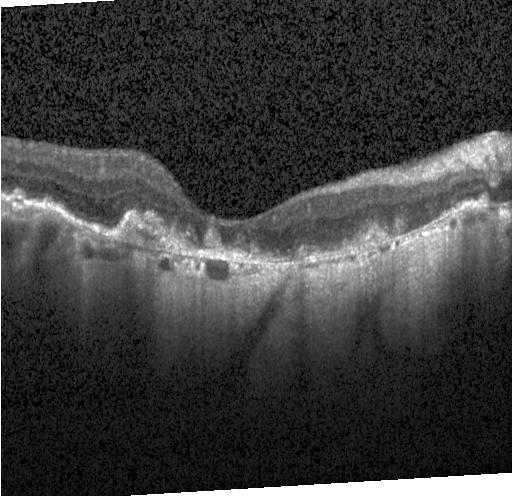 OCT B-scan · instrument: Heidelberg Spectralis · spectral-domain optical coherence tomography. This B-scan demonstrates choroidal neovascularization.